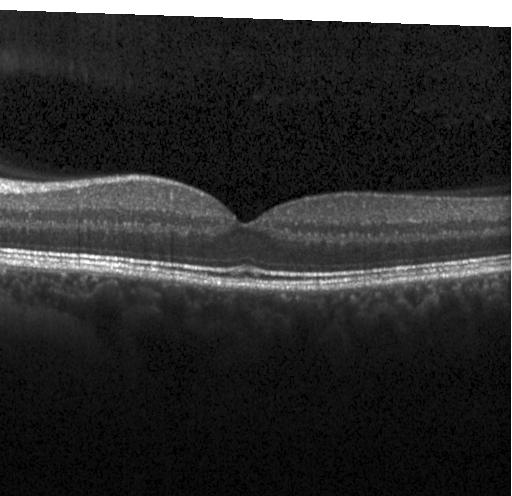

Optical coherence tomography scan; horizontal scan through the fovea.
Impression: no choroidal neovascularization, no diabetic macular edema, and no drusen.